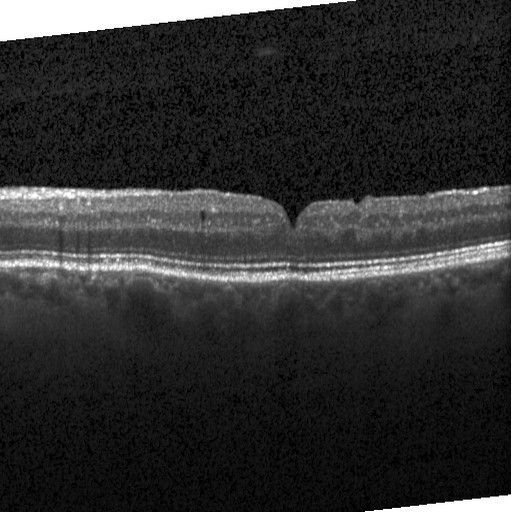
Retinal OCT cross-section. Acquired on a Heidelberg Spectralis
Diagnosis: diabetic macular edema (DME).